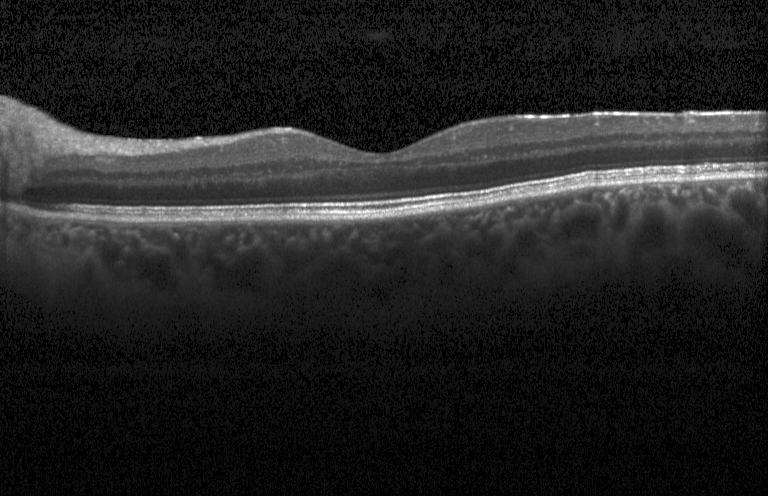 Retinal OCT B-scan. Diagnosis: neither choroidal neovascularization, diabetic macular edema, nor drusen.